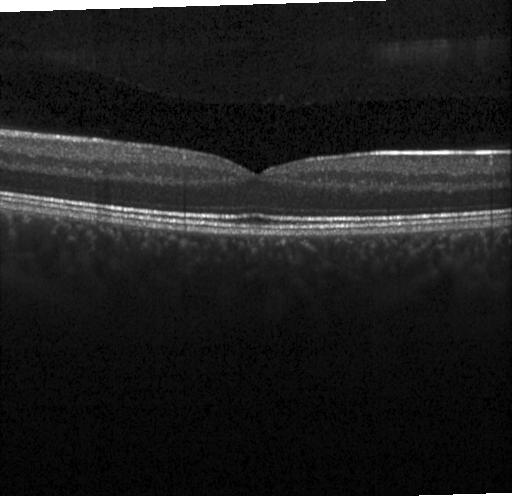
Finding: no choroidal neovascularization, no diabetic macular edema, and no drusen.